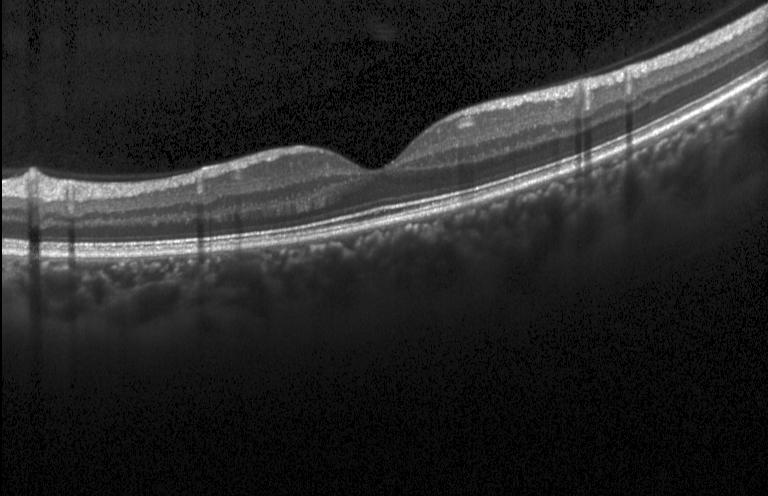 Diagnosis: no choroidal neovascularization, diabetic macular edema, or drusen.